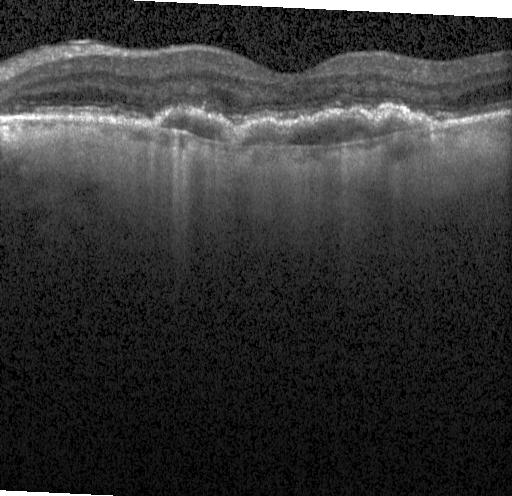
Optical coherence tomography scan. SD-OCT. Heidelberg Spectralis OCT system. Macular scan.
Impression: a choroidal neovascular membrane.